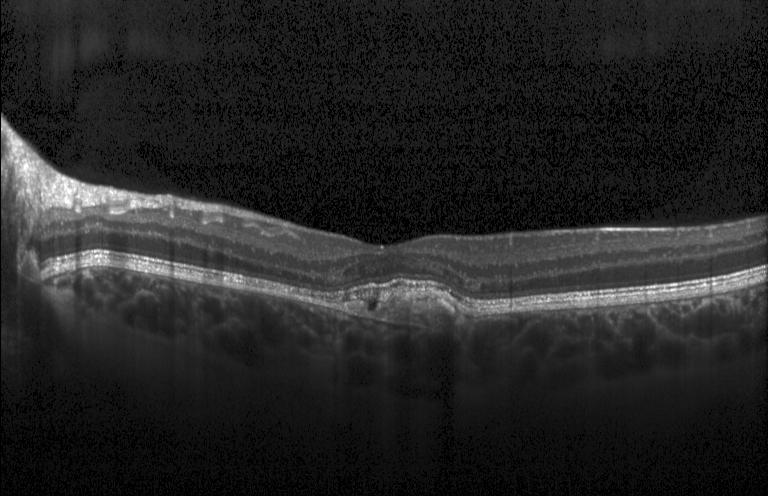 Retinal OCT cross-section. Heidelberg Spectralis OCT system
Finding: a choroidal neovascular membrane.